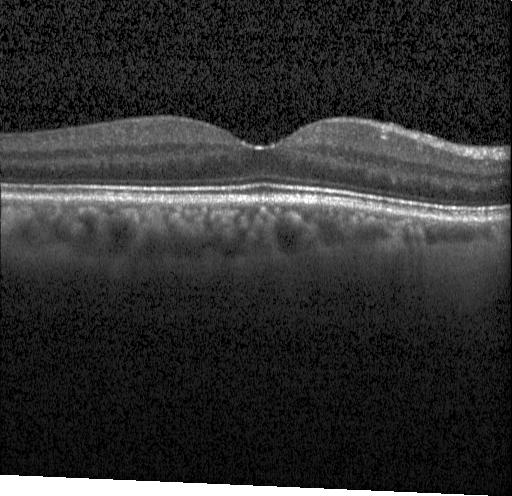 The scan shows neither choroidal neovascularization, diabetic macular edema, nor drusen.